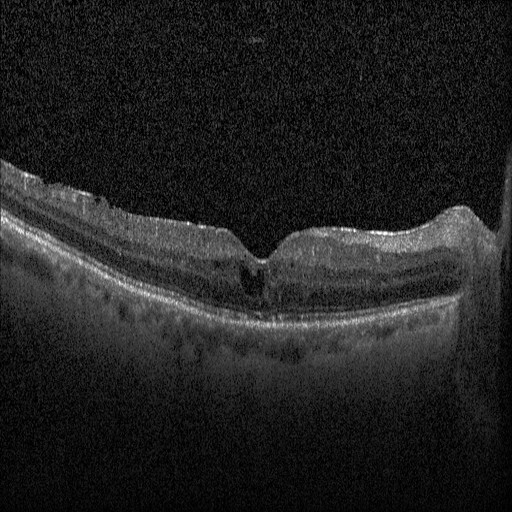 Optical coherence tomography B-scan. The scan shows DME.